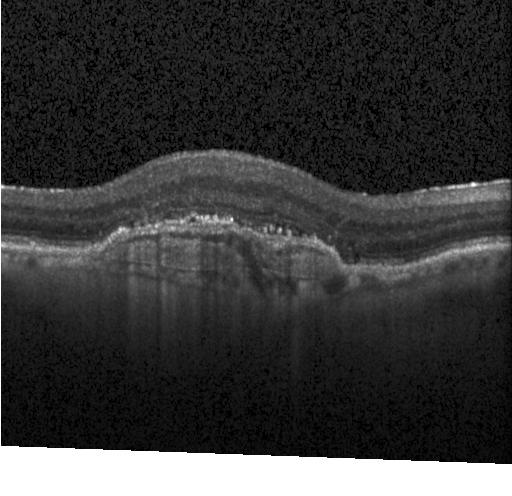

OCT B-scan
Choroidal neovascularization.